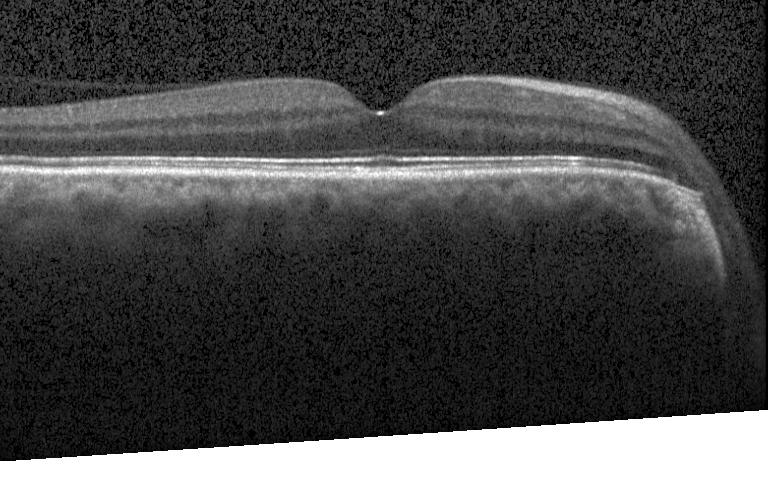

Through the macula; spectral-domain OCT; optical coherence tomography B-scan
Macular OCT: no choroidal neovascularization, no diabetic macular edema, and no drusen.